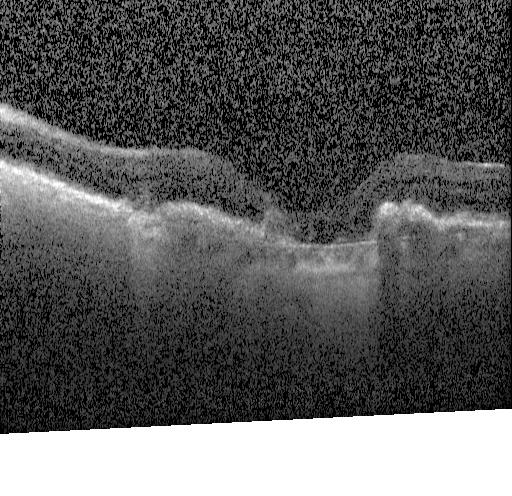
Fovea-centered; spectral-domain optical coherence tomography; Heidelberg Spectralis; retinal OCT B-scan — This B-scan demonstrates CNV.